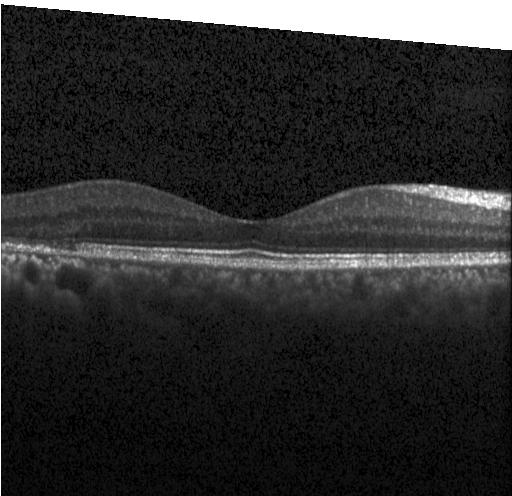

This B-scan demonstrates no choroidal neovascularization, diabetic macular edema, or drusen.